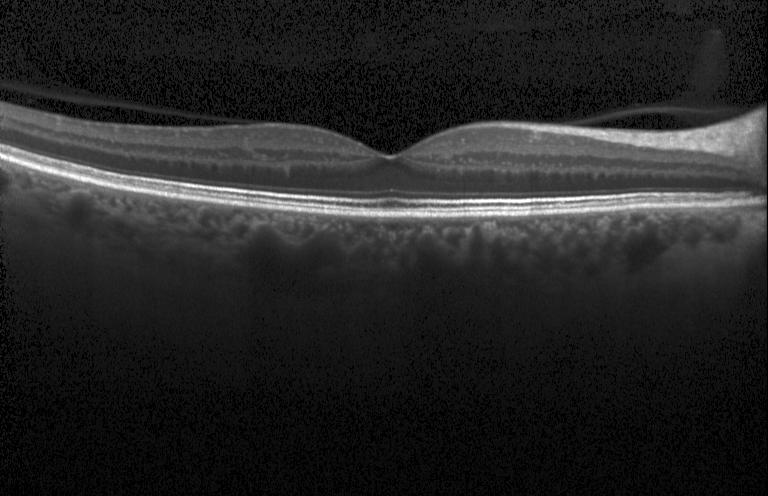

Diagnosis: neither CNV, DME, nor drusen.